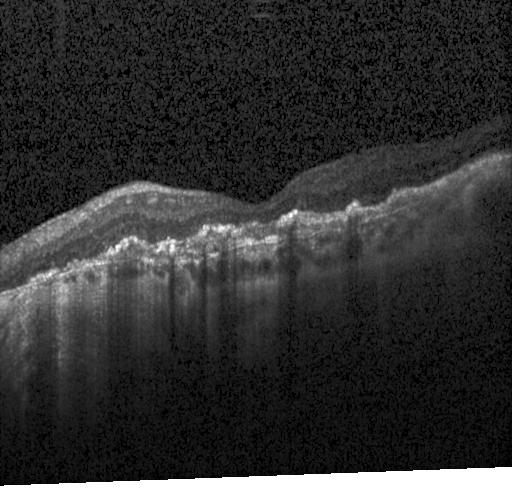

Retinal OCT B-scan — Macular OCT: a choroidal neovascular membrane.